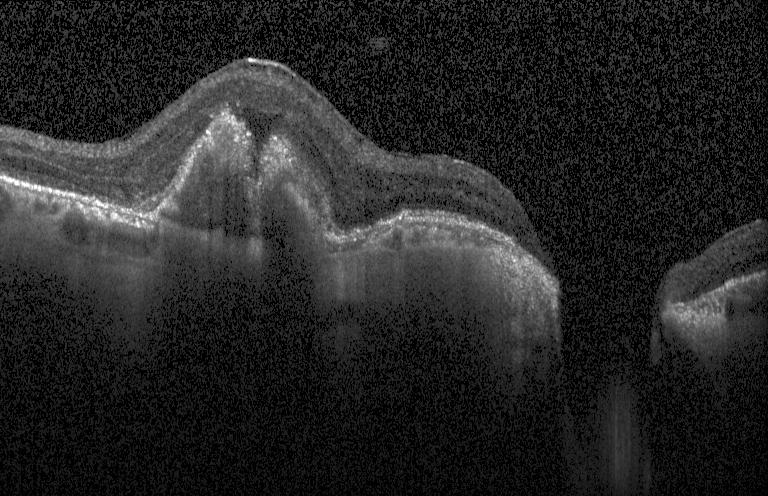
Dx: a choroidal neovascular membrane.